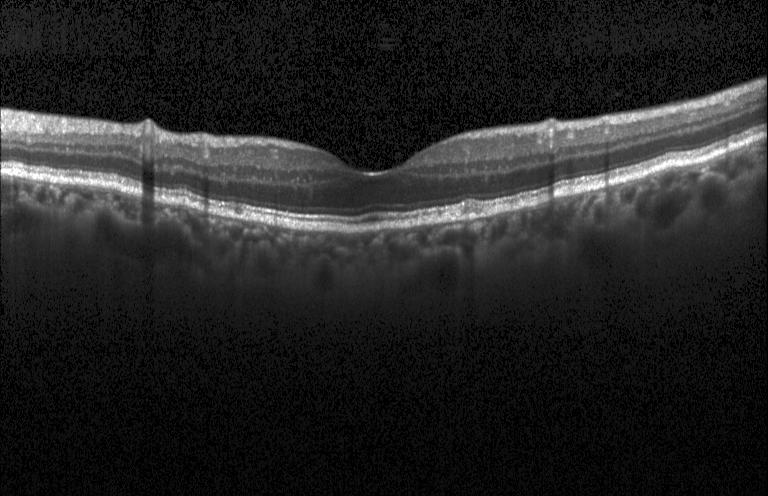 Spectral-domain OCT · macular scan · Heidelberg Spectralis · OCT B-scan
Diagnosis: sub-RPE drusenoid deposits.